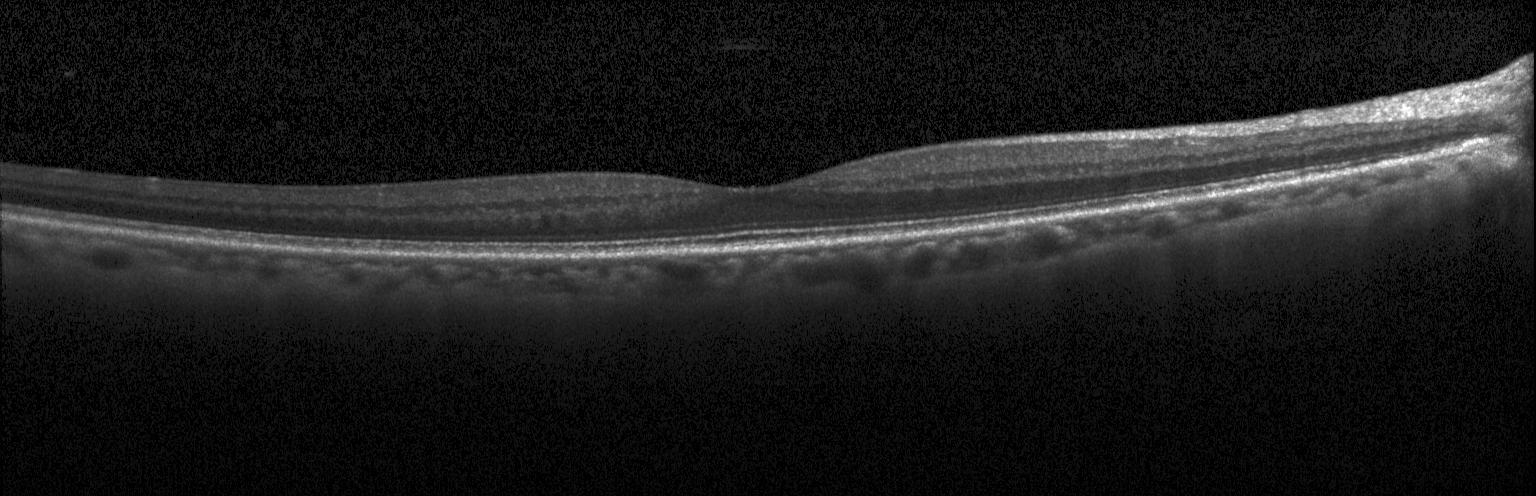 Diagnosis: neither choroidal neovascularization, diabetic macular edema, nor drusen.